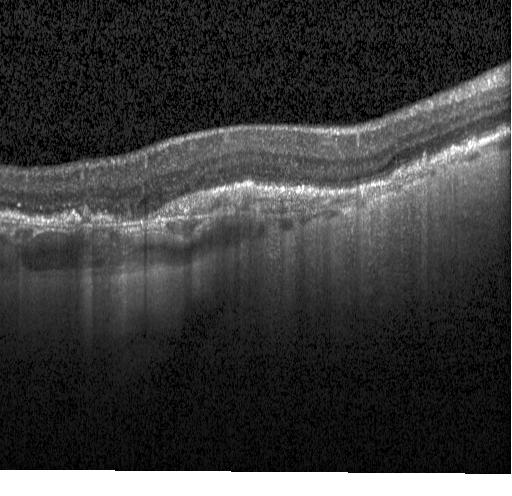

Optical coherence tomography B-scan
Assessment: choroidal neovascularization.